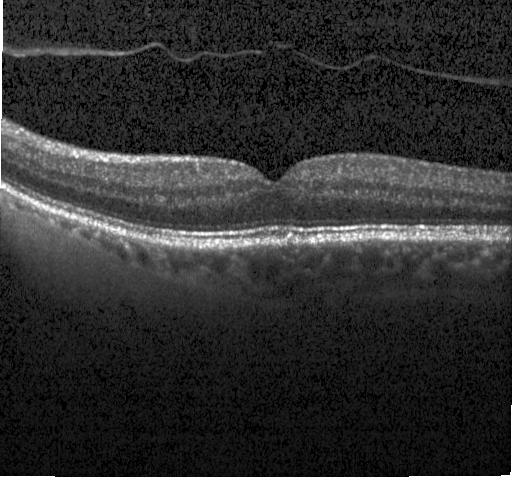
SD-OCT, retinal OCT B-scan, Heidelberg Spectralis.
Impression: drusen.